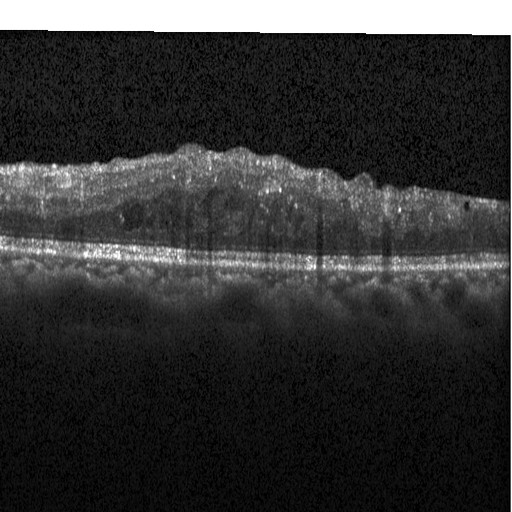

Retinal OCT B-scan. Fovea-centered. Heidelberg Spectralis OCT system. Spectral-domain optical coherence tomography — Macular OCT: DME.